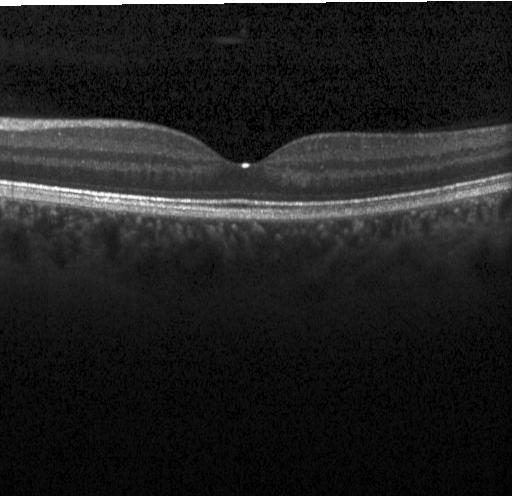

Acquired on a Heidelberg Spectralis · optical coherence tomography scan · centered on the fovea.
The scan shows no choroidal neovascularization, no diabetic macular edema, and no drusen.